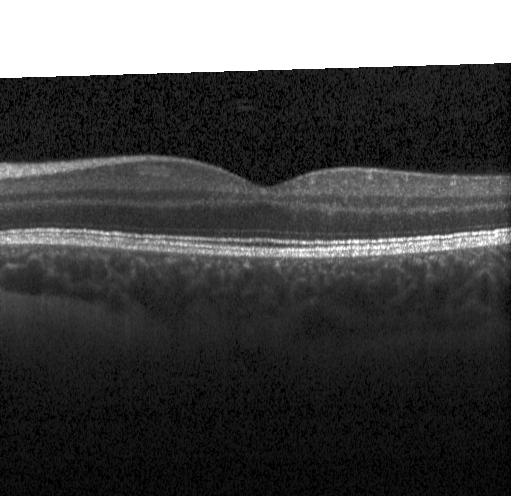 Heidelberg Spectralis · optical coherence tomography B-scan.
This B-scan demonstrates no choroidal neovascularization, no diabetic macular edema, and no drusen.